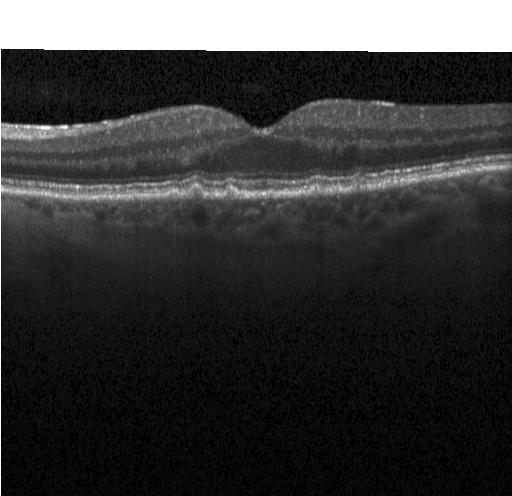
Retinal OCT cross-section
Diagnosis: sub-RPE drusenoid deposits.